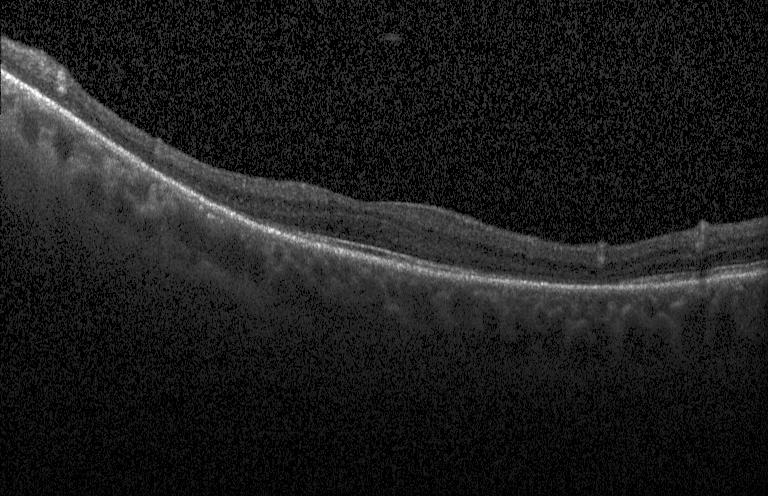

Optical coherence tomography B-scan.
Assessment: neither choroidal neovascularization, diabetic macular edema, nor drusen.